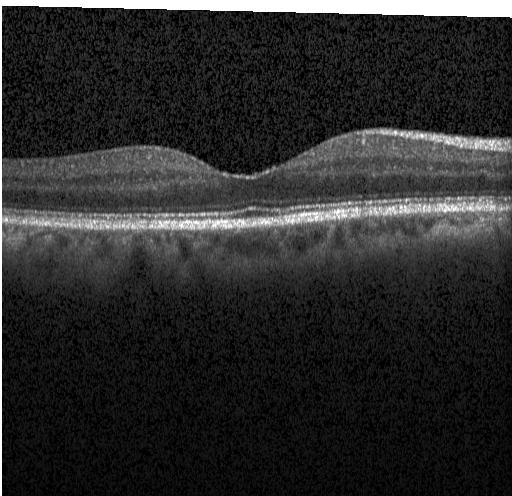

Heidelberg Spectralis OCT system; retinal OCT cross-section
Macular OCT: no CNV, DME, or drusen.